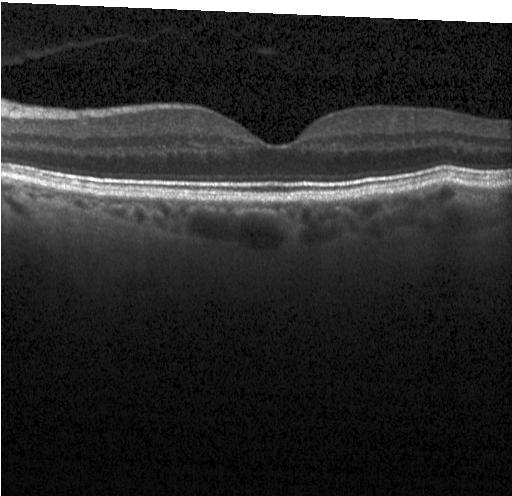

OCT line scan
Finding: no evidence of CNV, DME, or drusen.